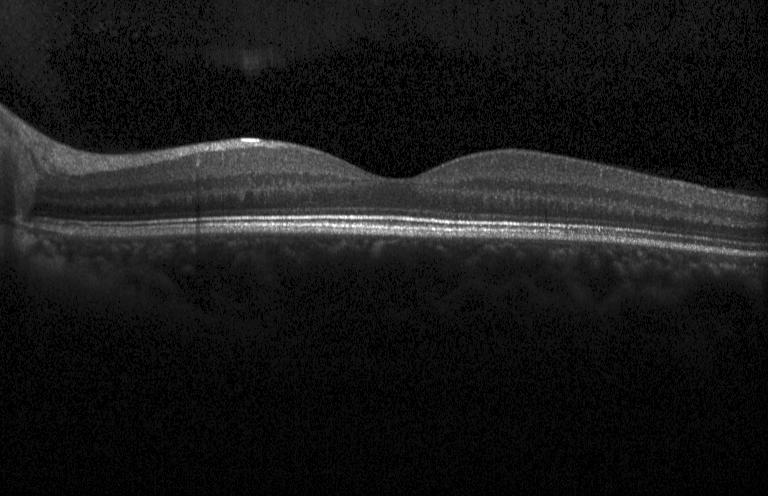
Optical coherence tomography scan; instrument: Heidelberg Spectralis. Impression: neither choroidal neovascularization, diabetic macular edema, nor drusen.